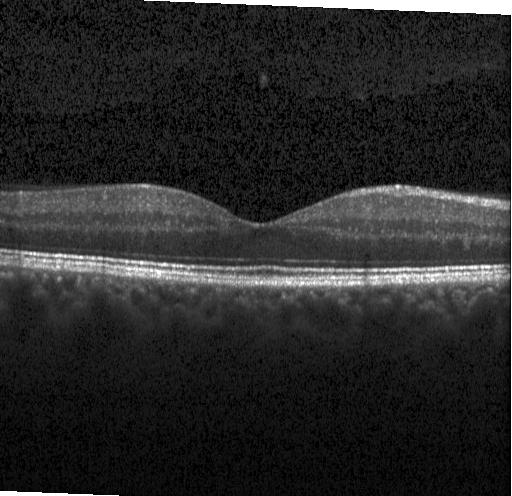

Optical coherence tomography B-scan.
Assessment: no CNV, no DME, and no drusen.